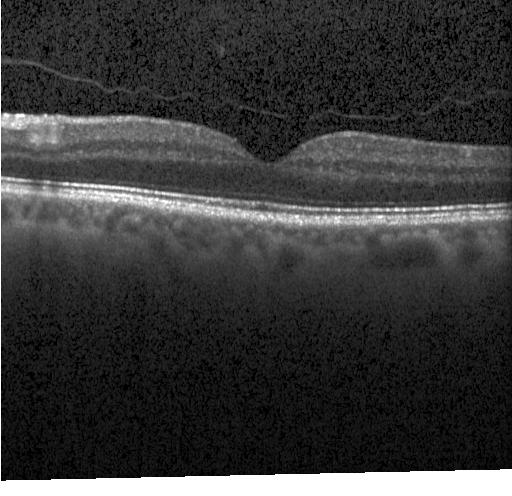
Centered on the fovea, retinal OCT cross-section.
Macular OCT: neither CNV, DME, nor drusen.